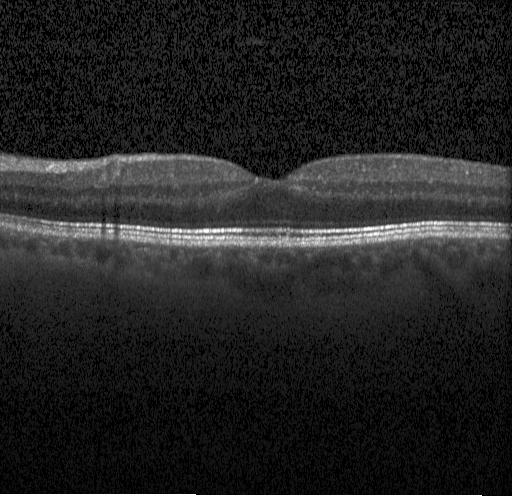

Assessment: no CNV, DME, or drusen.